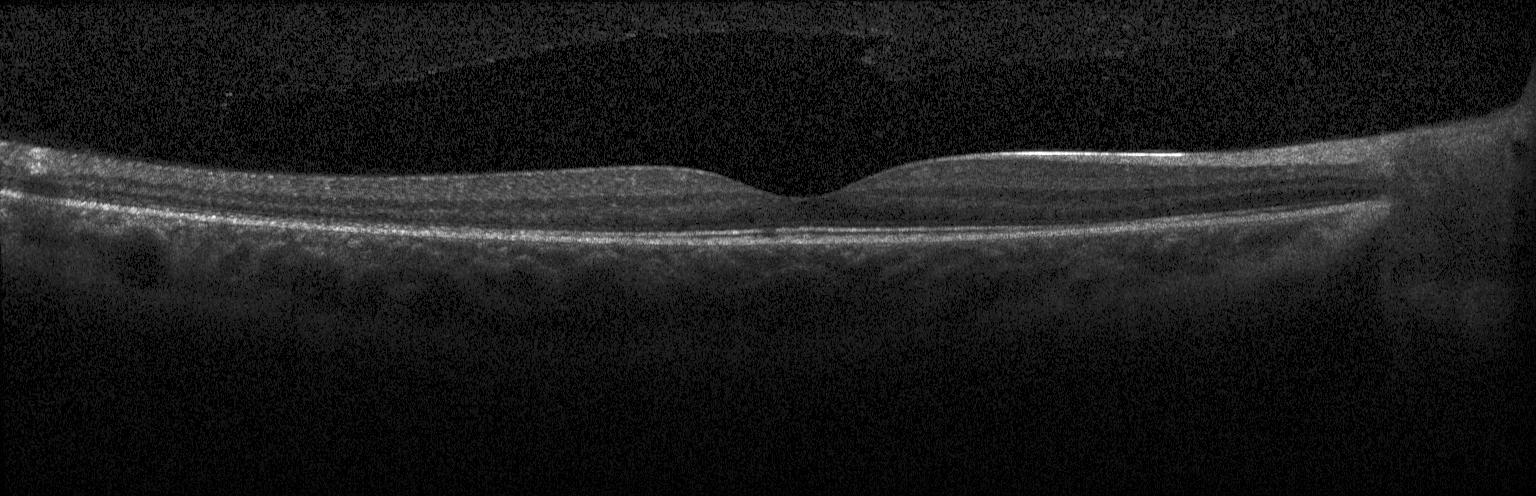

Instrument: Heidelberg Spectralis; retinal OCT cross-section; spectral-domain optical coherence tomography. The scan shows no choroidal neovascularization, no diabetic macular edema, and no drusen.